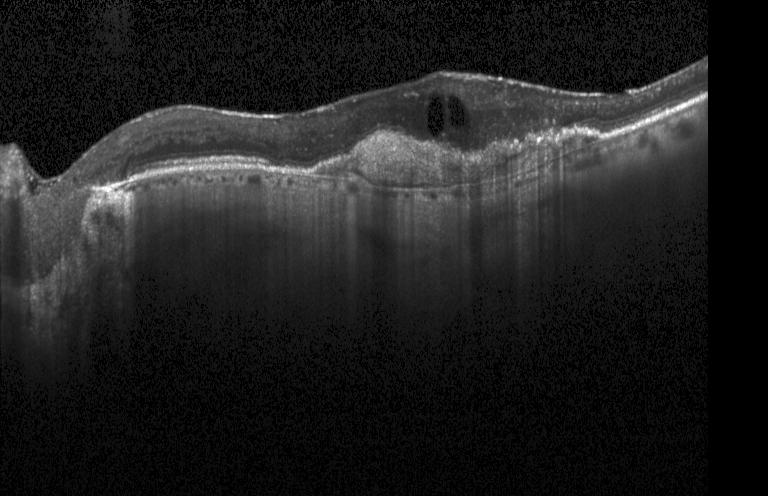
SD-OCT · fovea-centered · retinal OCT B-scan · instrument: Heidelberg Spectralis
This B-scan demonstrates choroidal neovascularization.